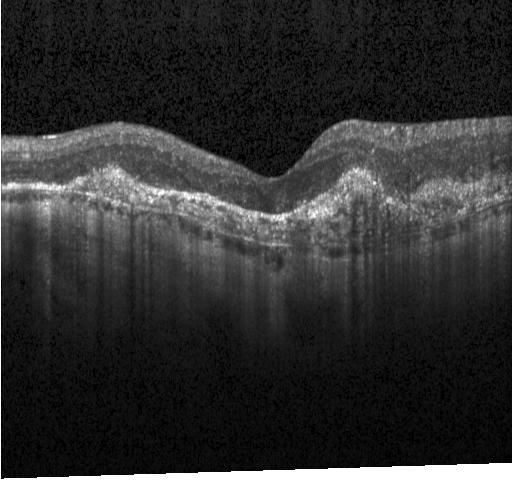

OCT line scan
Diagnosis: a choroidal neovascular membrane.